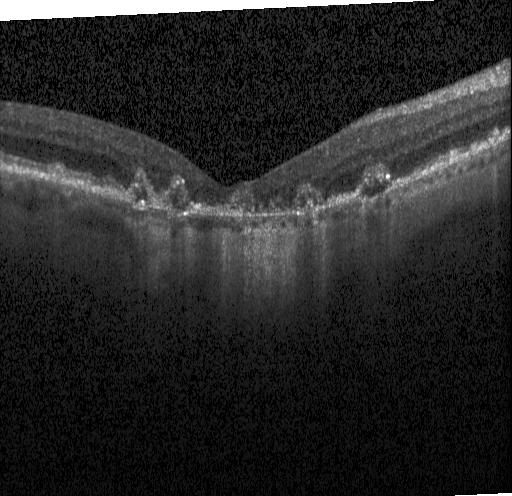
OCT B-scan — Macular OCT: choroidal neovascularization.